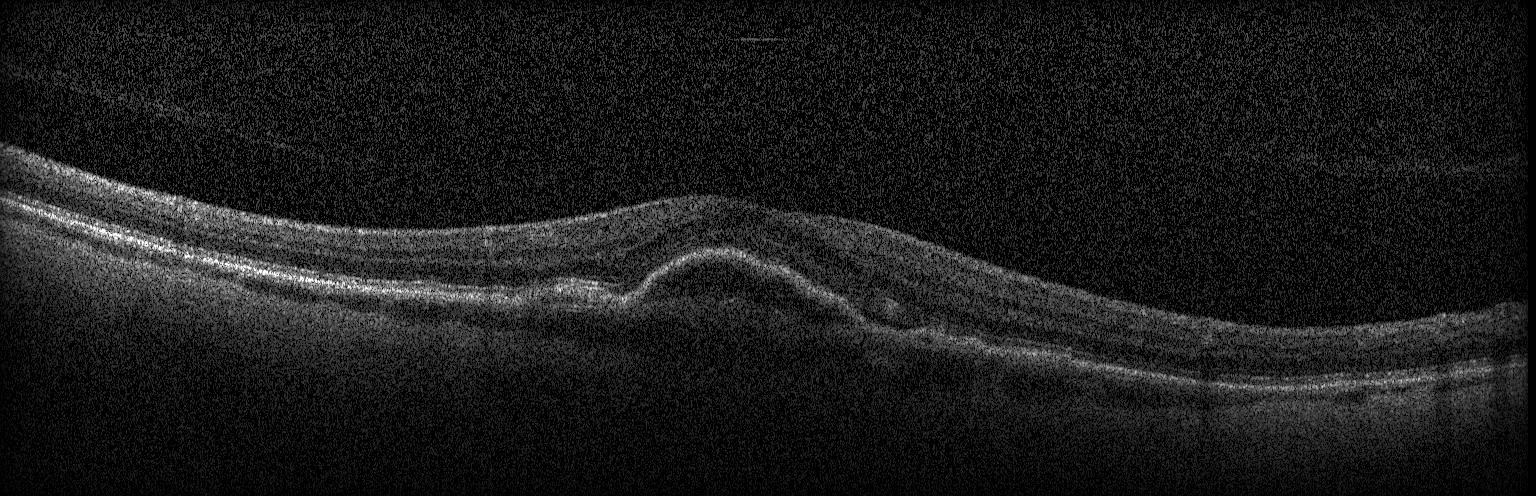 Centered on the fovea · OCT line scan — Diagnosis: CNV.